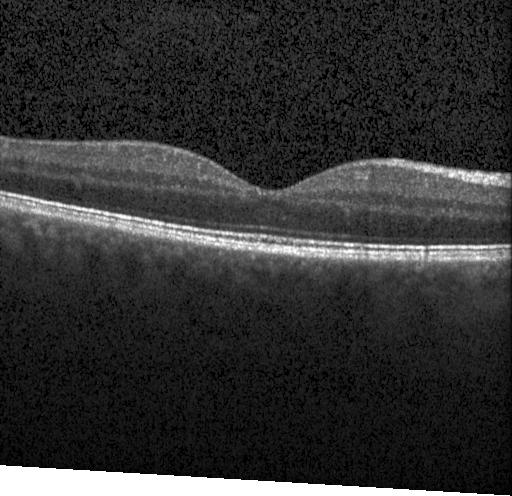

OCT line scan · Heidelberg Spectralis. No evidence of choroidal neovascularization, diabetic macular edema, or drusen.